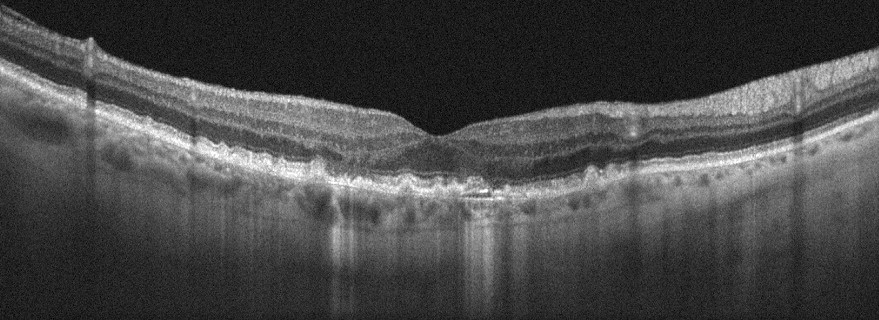
Spectral-domain OCT B-scan: age-related macular degeneration.